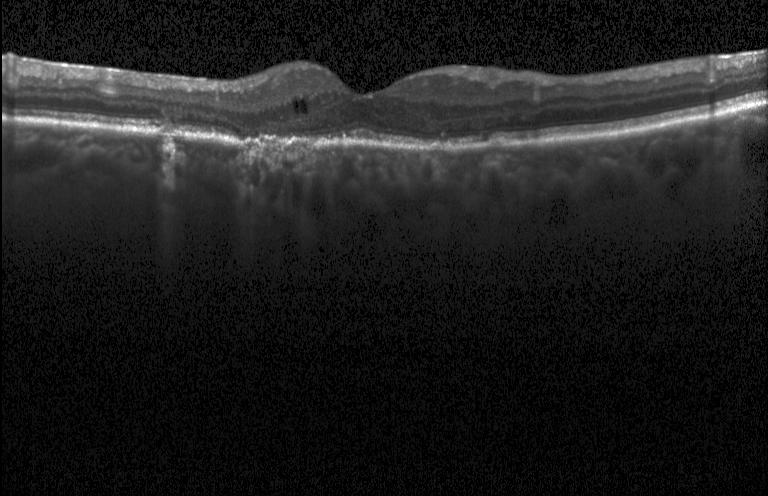 OCT B-scan.
Macular OCT: a choroidal neovascular membrane.